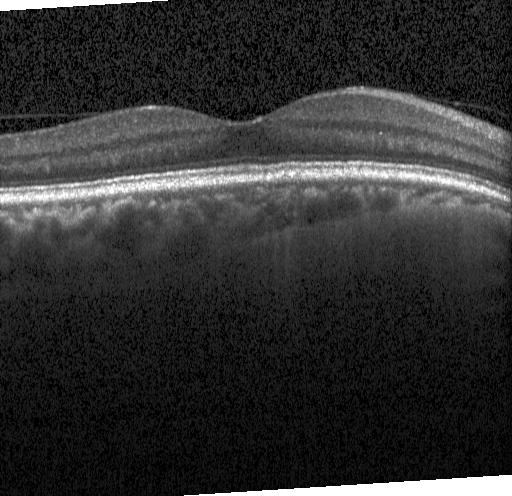 OCT scan showing neither choroidal neovascularization, diabetic macular edema, nor drusen.